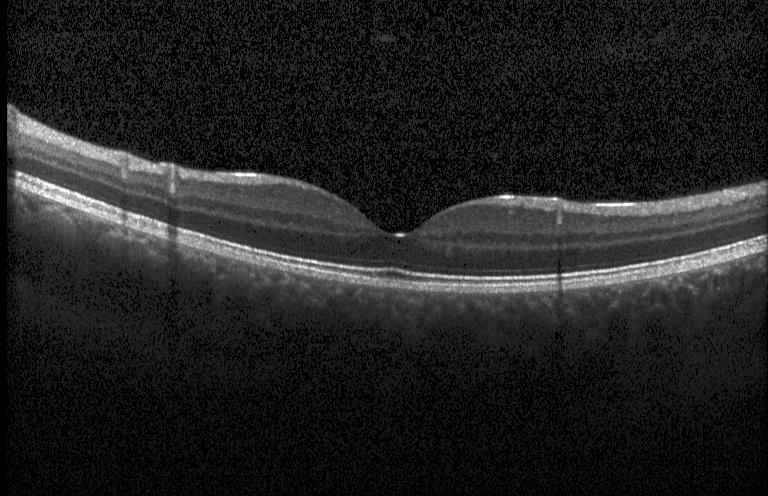 This B-scan demonstrates no CNV, no DME, and no drusen.